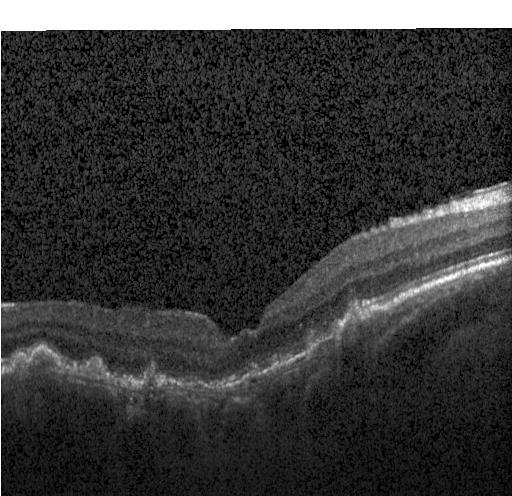 OCT B-scan — CNV.